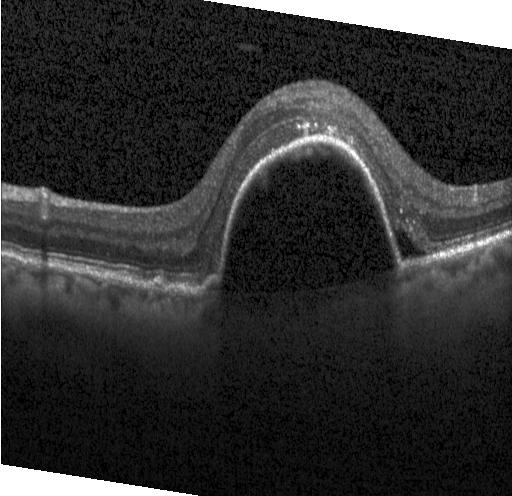 Optical coherence tomography scan. Impression: choroidal neovascularization.